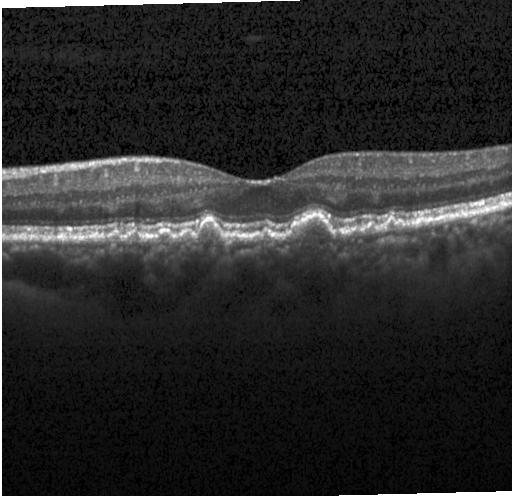 Heidelberg Spectralis; spectral-domain optical coherence tomography; retinal OCT B-scan; through the macula. This B-scan demonstrates sub-RPE drusenoid deposits.